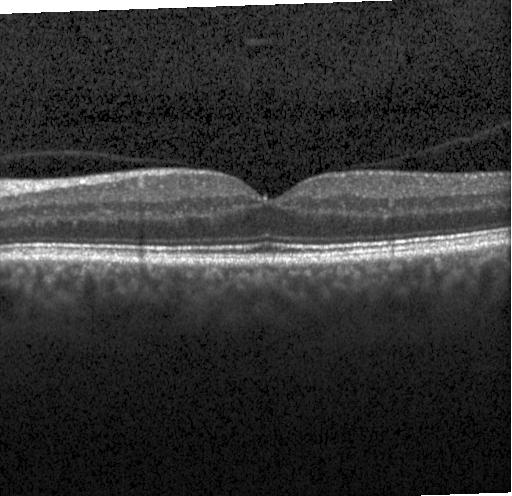 Optical coherence tomography B-scan — Diagnosis: no choroidal neovascularization, diabetic macular edema, or drusen.